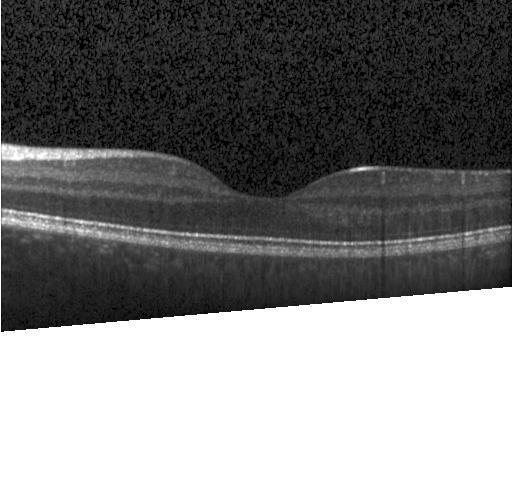

Spectral-domain OCT. Optical coherence tomography scan. Acquired on a Heidelberg Spectralis — Impression: neither choroidal neovascularization, diabetic macular edema, nor drusen.